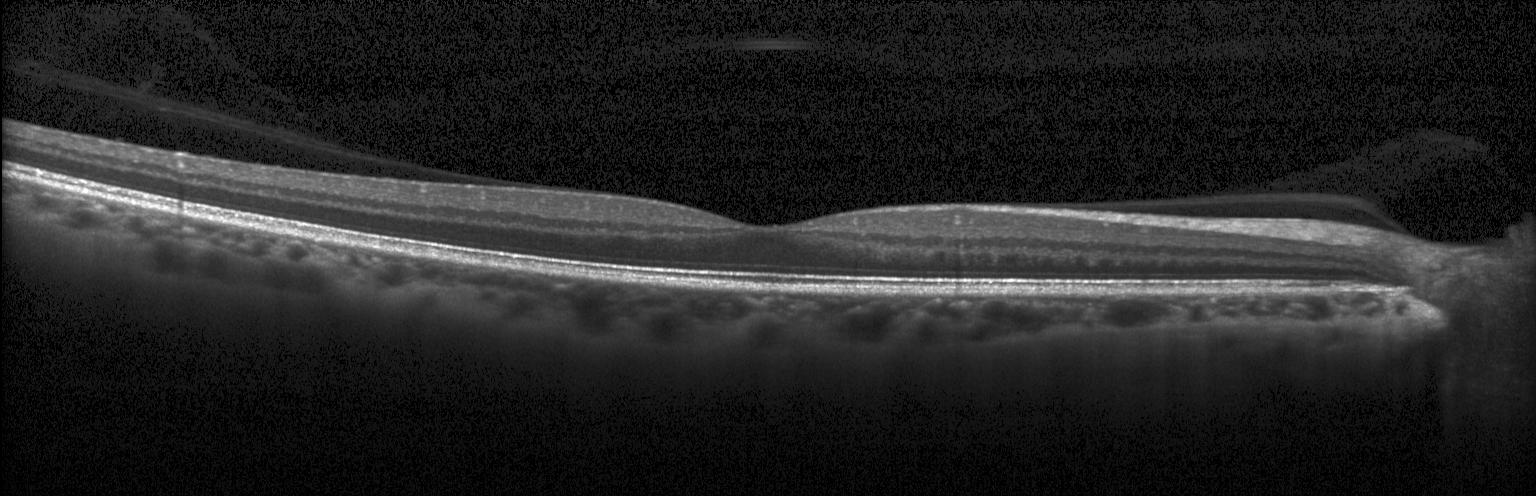

OCT line scan. Macular scan
Finding: no choroidal neovascularization, diabetic macular edema, or drusen.